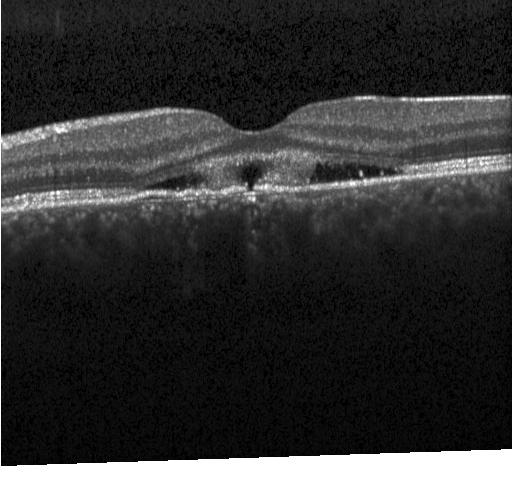 Impression: a choroidal neovascular membrane.